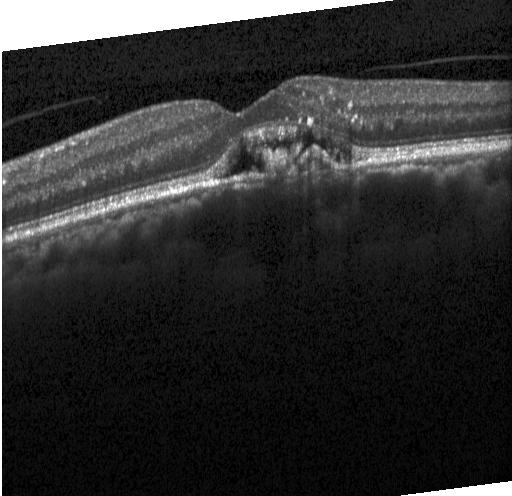 Spectral-domain OCT. Acquired on a Heidelberg Spectralis. Through the macula. OCT B-scan
The scan shows a choroidal neovascular membrane.